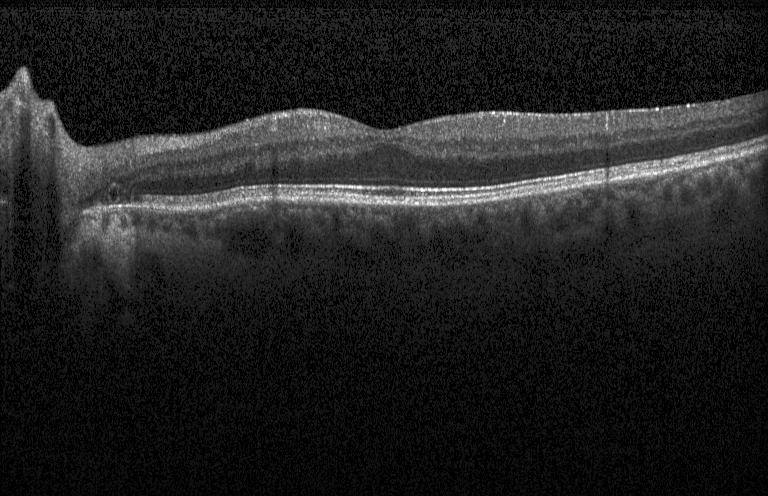 Heidelberg Spectralis OCT system, SD-OCT, retinal OCT B-scan.
Impression: no choroidal neovascularization, no diabetic macular edema, and no drusen.